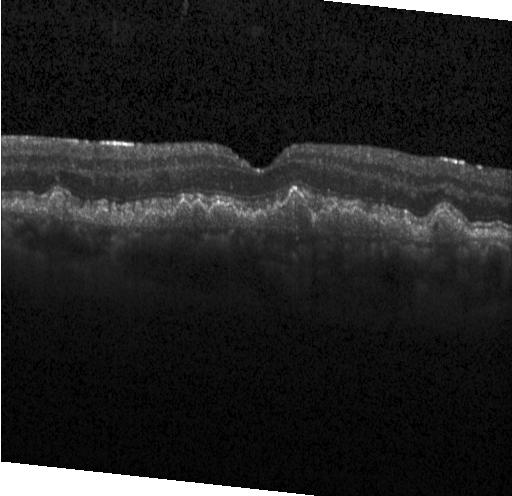
Finding: CNV.